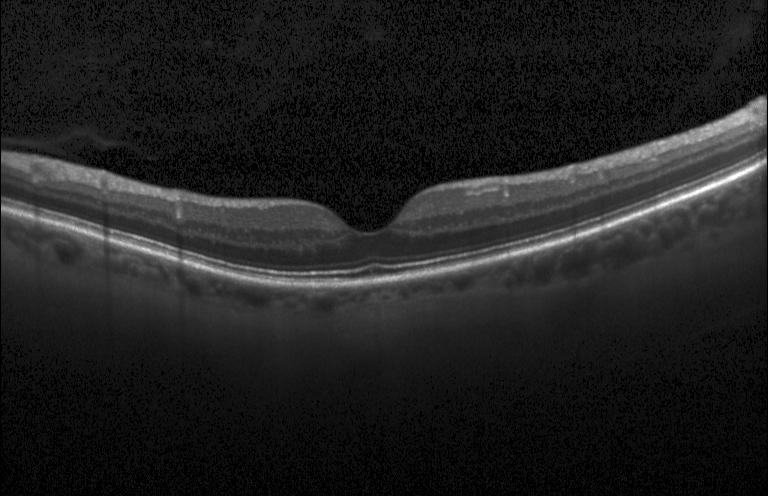 Horizontal scan through the fovea. Spectral-domain OCT. OCT line scan. Acquired on a Heidelberg Spectralis
The scan shows no choroidal neovascularization, no diabetic macular edema, and no drusen.